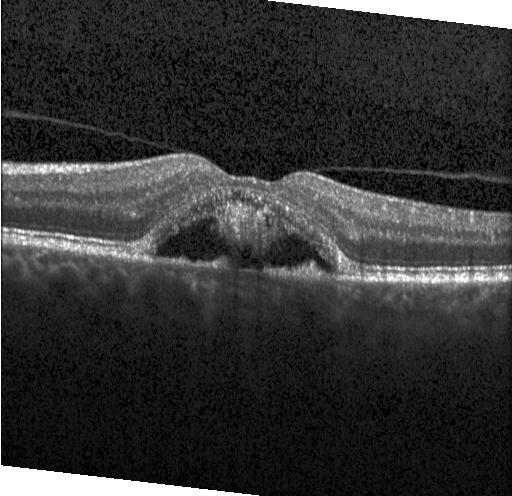
Instrument: Heidelberg Spectralis; optical coherence tomography B-scan; horizontal scan through the fovea; spectral-domain OCT. Impression: a choroidal neovascular membrane.